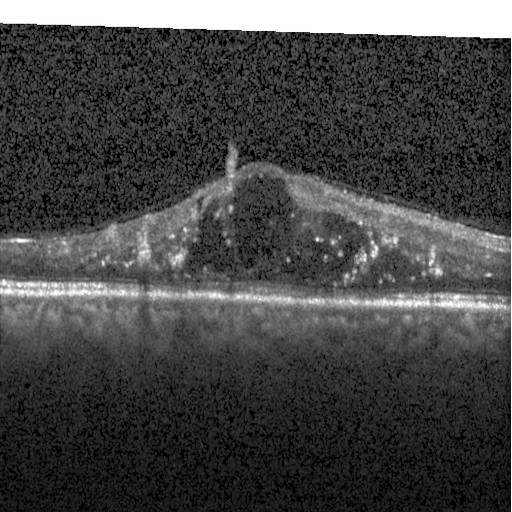 The scan shows diabetic macular edema.